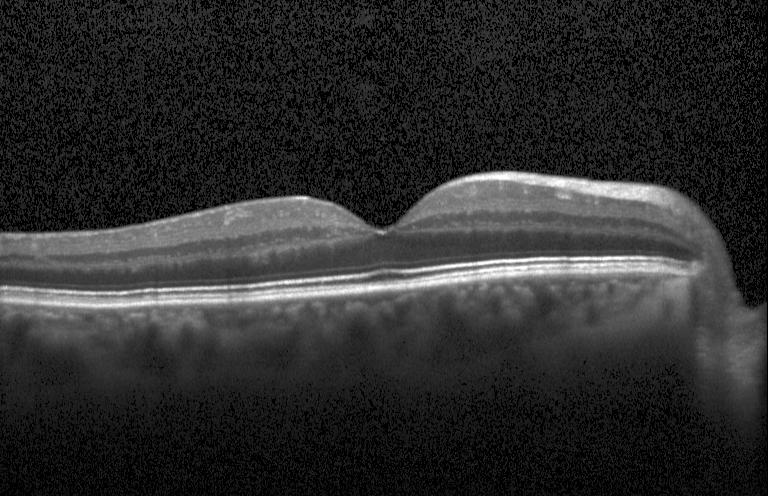
Retinal OCT cross-section; SD-OCT
Diagnosis: no evidence of CNV, DME, or drusen.